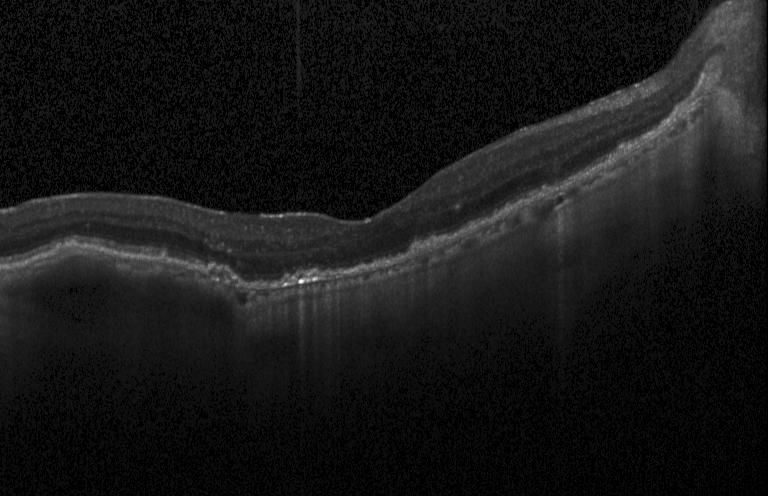 Retinal OCT cross-section showing a choroidal neovascular membrane.